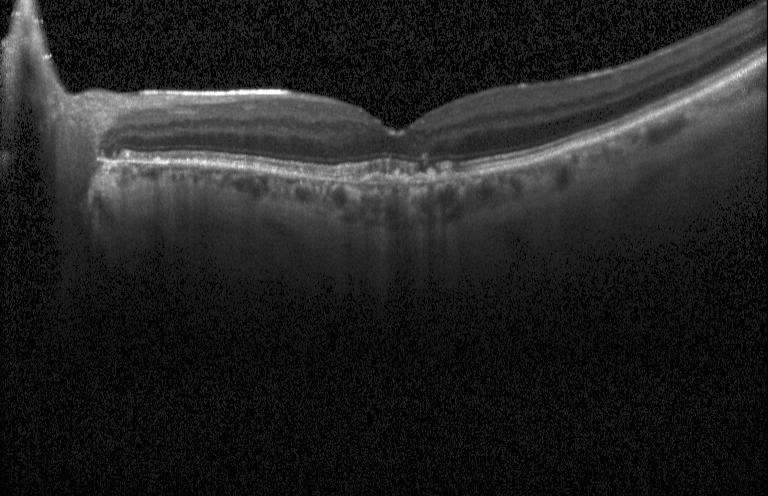
Spectral-domain optical coherence tomography; Heidelberg Spectralis OCT system; optical coherence tomography scan; fovea-centered.
Diagnosis: a choroidal neovascular membrane.